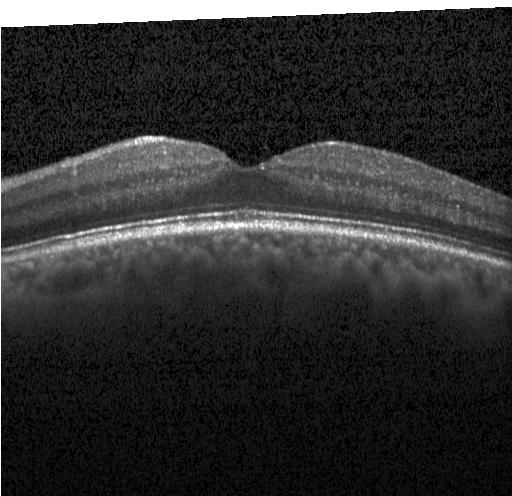
The scan shows no evidence of CNV, DME, or drusen.